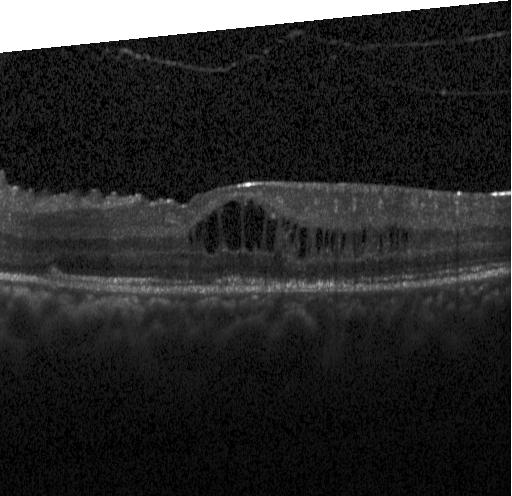 Retinal OCT cross-section, spectral-domain optical coherence tomography, through the macula, acquired on a Heidelberg Spectralis. OCT finding: DME.